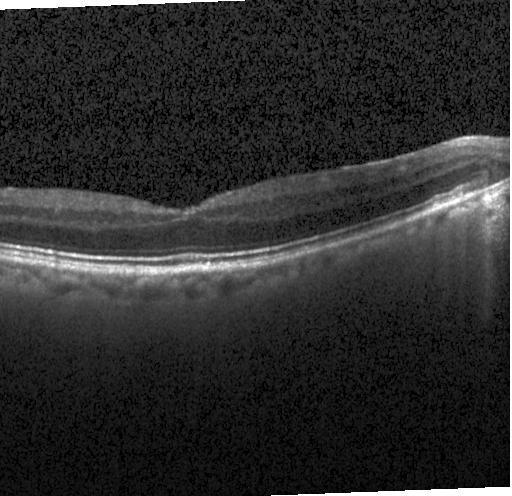
OCT line scan. Horizontal scan through the fovea.
This B-scan demonstrates no CNV, DME, or drusen.